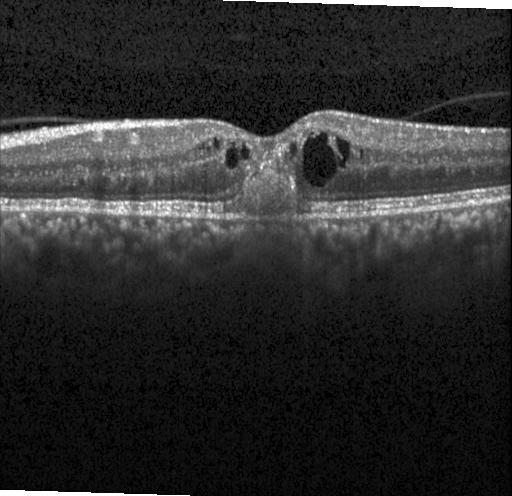 SD-OCT · acquired on a Heidelberg Spectralis · optical coherence tomography scan · centered on the fovea
A choroidal neovascular membrane.